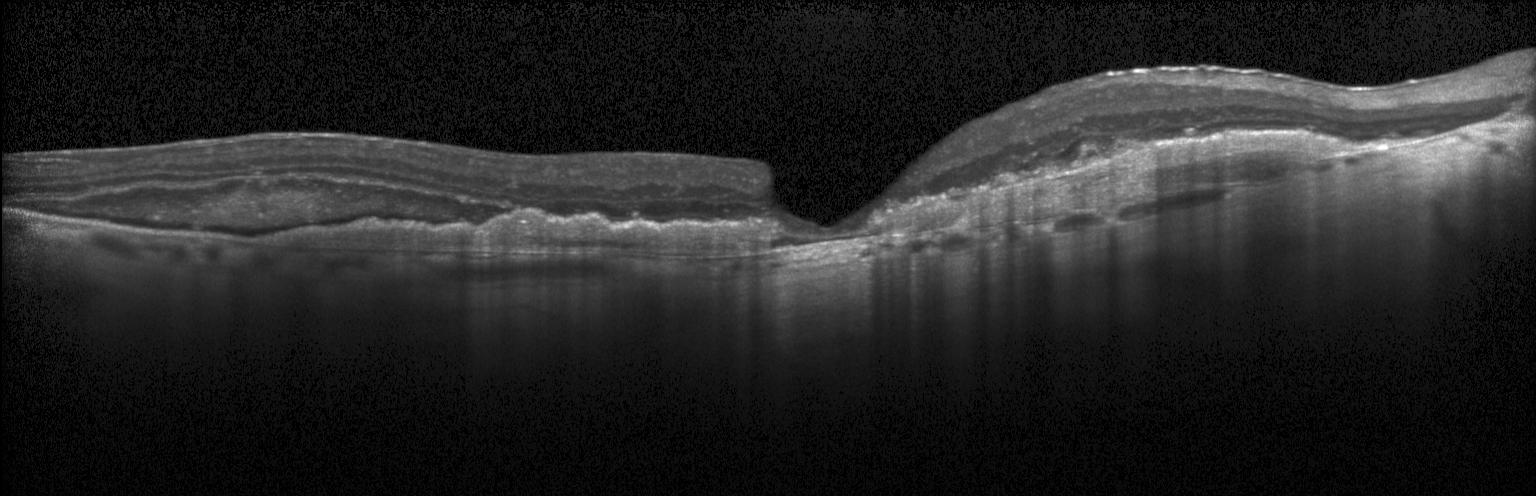
Heidelberg Spectralis OCT system; through the macula; retinal OCT B-scan
Assessment: a choroidal neovascular membrane.